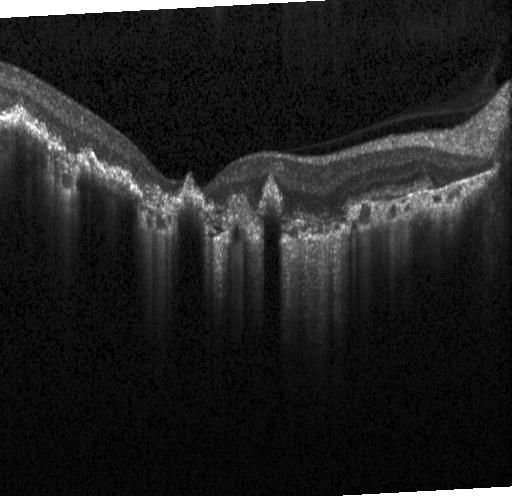 OCT finding: a choroidal neovascular membrane.